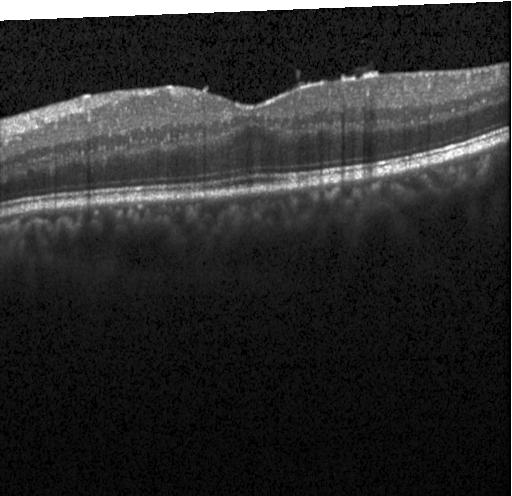
OCT B-scan
No choroidal neovascularization, no diabetic macular edema, and no drusen.